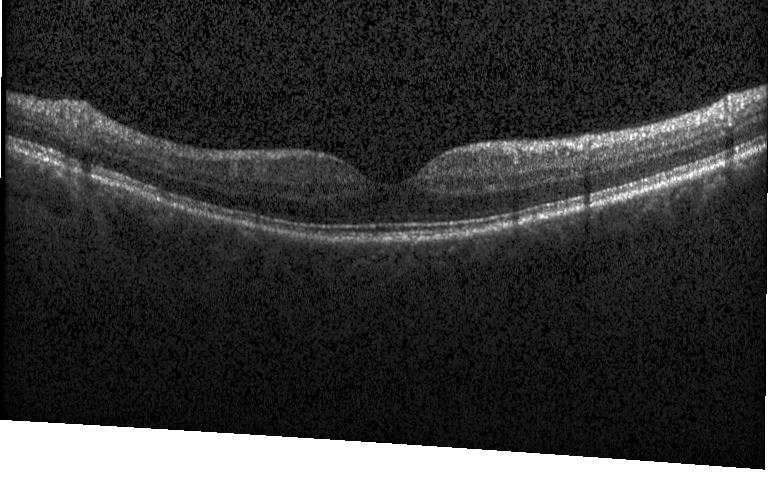

Retinal OCT cross-section showing no choroidal neovascularization, diabetic macular edema, or drusen.